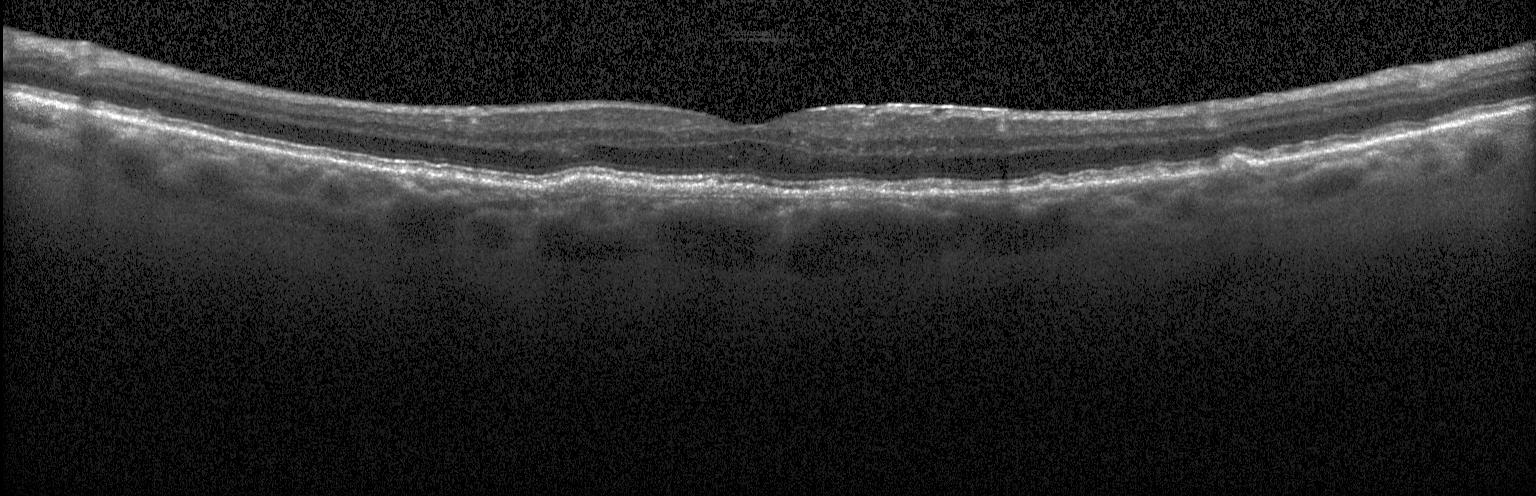

Finding: a choroidal neovascular membrane.